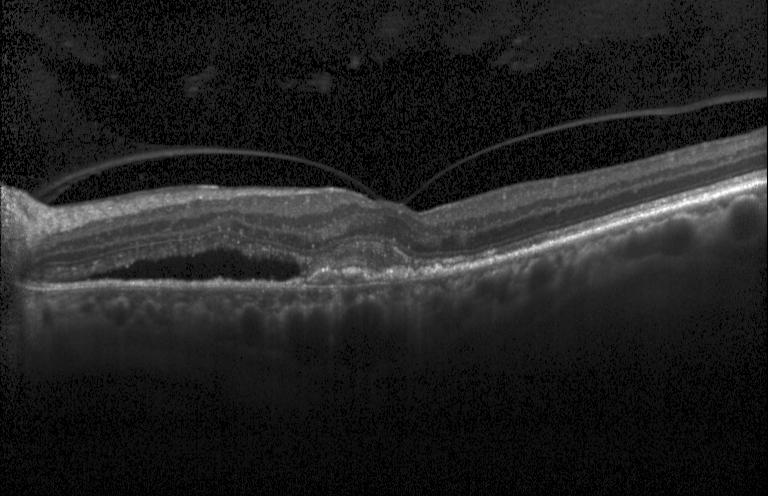 Retinal OCT cross-section showing CNV.